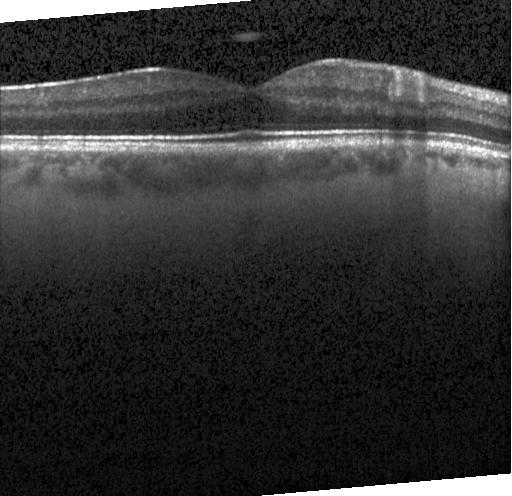

Optical coherence tomography scan; Heidelberg Spectralis OCT system.
Diagnosis: no evidence of choroidal neovascularization, diabetic macular edema, or drusen.